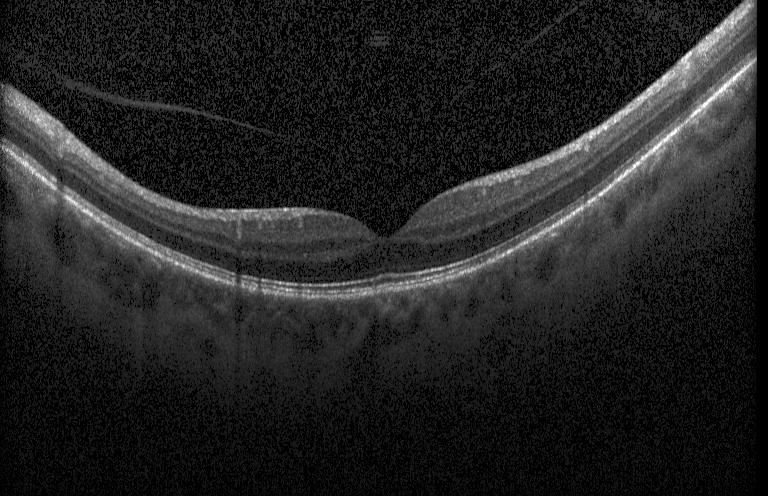 Spectral-domain OCT. Heidelberg Spectralis. OCT B-scan. Finding: no CNV, no DME, and no drusen.